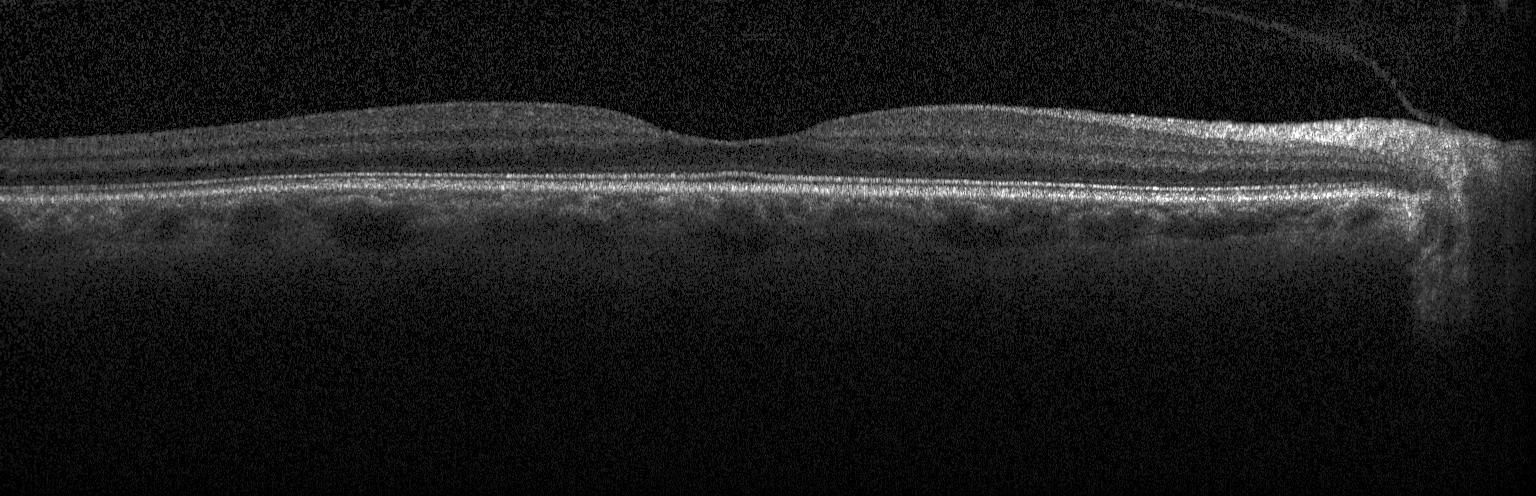 Spectral-domain OCT B-scan: no CNV, no DME, and no drusen.